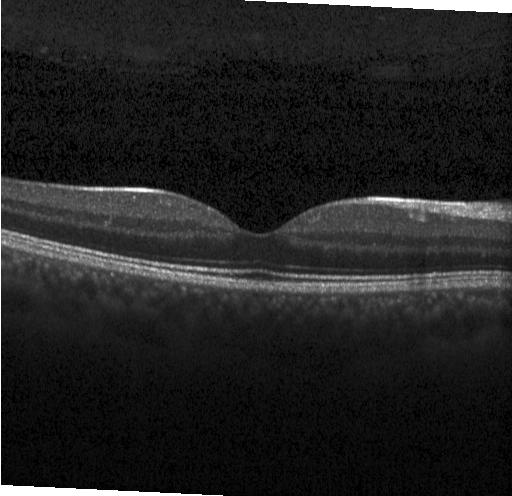 OCT line scan.
OCT finding: no choroidal neovascularization, diabetic macular edema, or drusen.